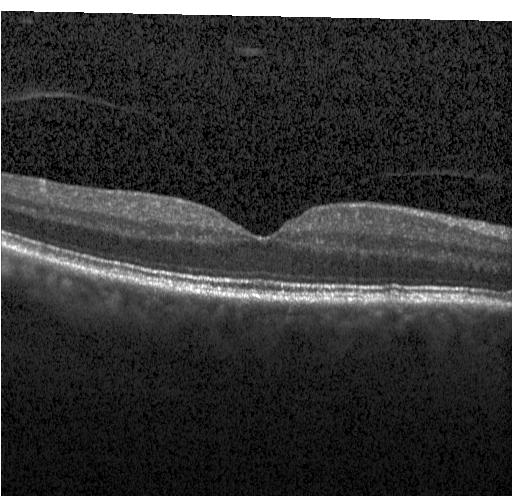
OCT B-scan — Diagnosis: neither choroidal neovascularization, diabetic macular edema, nor drusen.